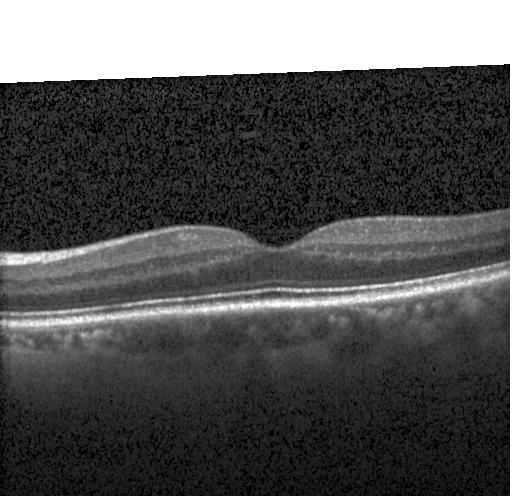 OCT B-scan showing no choroidal neovascularization, no diabetic macular edema, and no drusen.